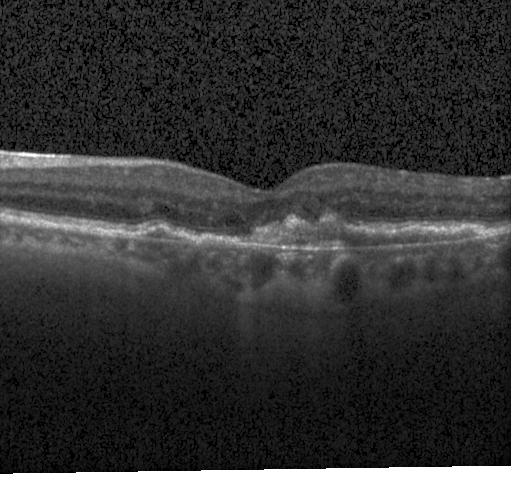

OCT line scan
Finding: a choroidal neovascular membrane.